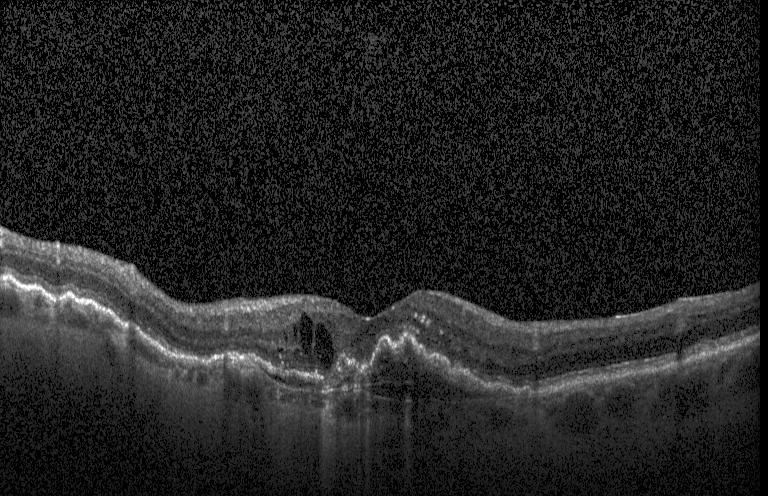 OCT B-scan; instrument: Heidelberg Spectralis — OCT finding: a choroidal neovascular membrane.